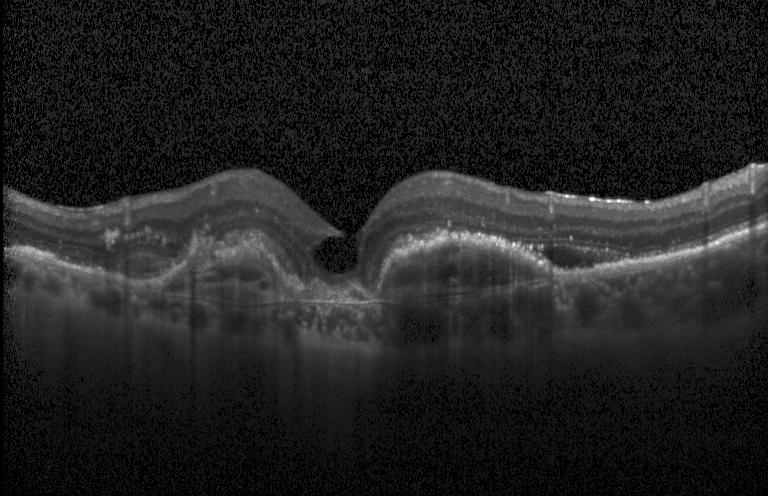
Finding: CNV.